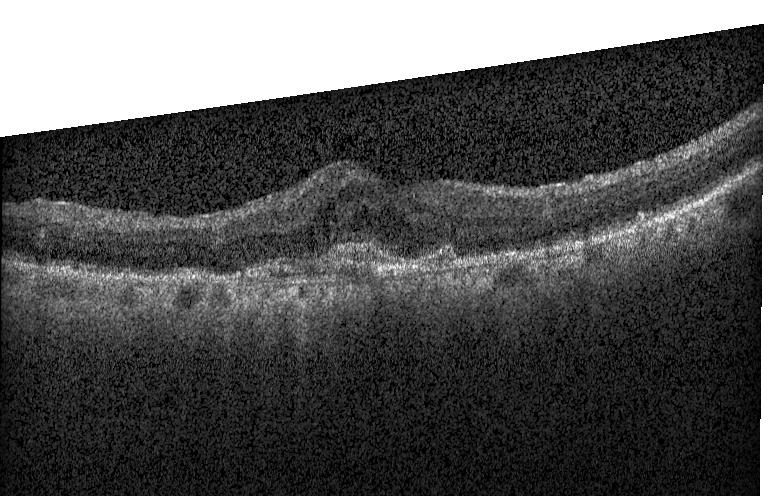 Finding: choroidal neovascularization (CNV).